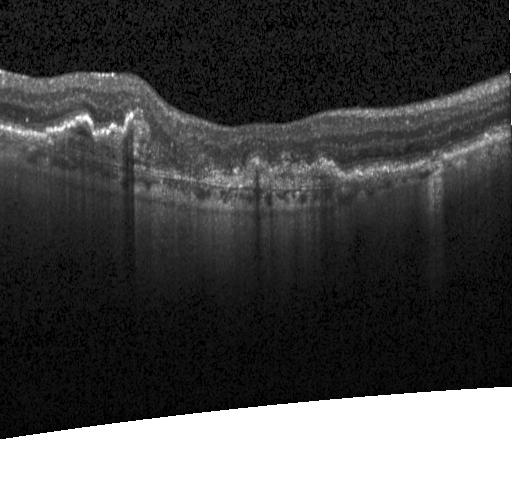 Instrument: Heidelberg Spectralis. Spectral-domain OCT. Optical coherence tomography scan — Impression: CNV.